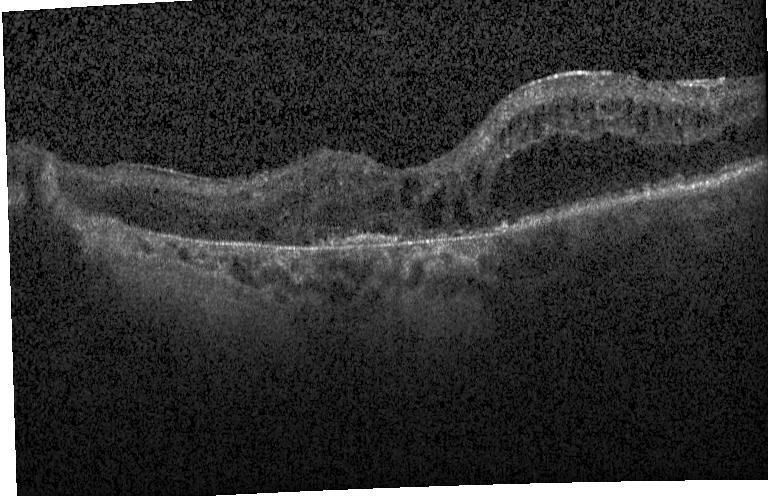

Spectral-domain optical coherence tomography, acquired on a Heidelberg Spectralis, optical coherence tomography scan
Diagnosis: CNV.